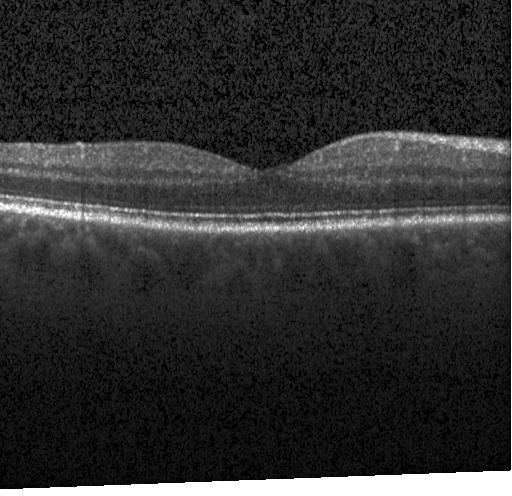

Diagnosis: no evidence of choroidal neovascularization, diabetic macular edema, or drusen.